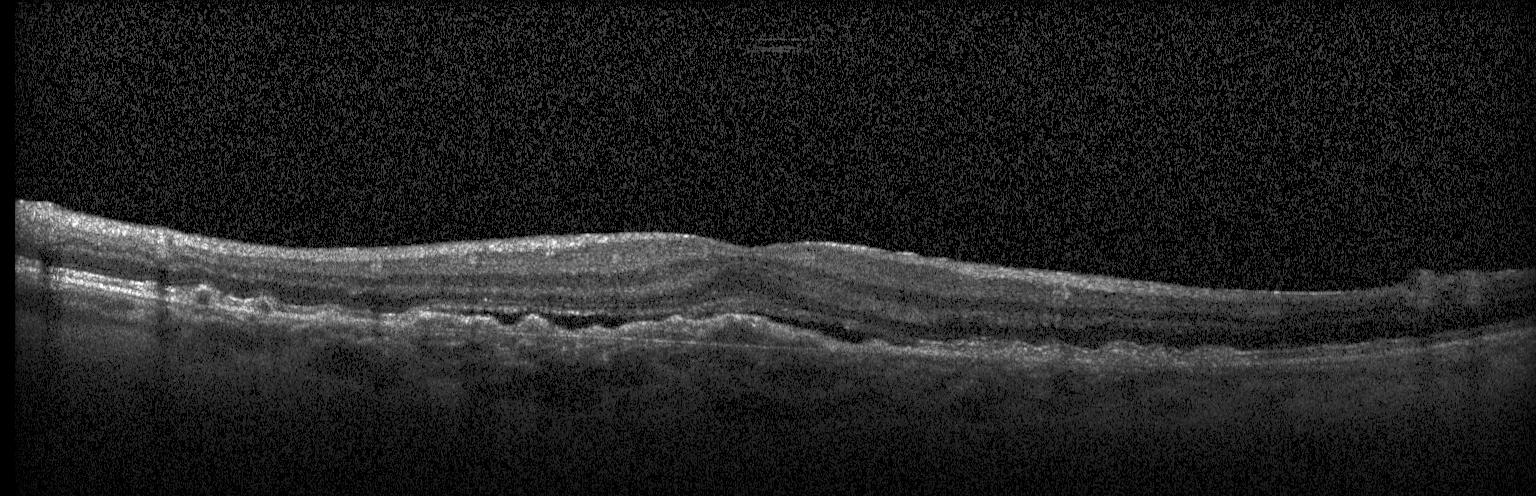
Through the macula; SD-OCT; optical coherence tomography B-scan; Heidelberg Spectralis
Finding: a choroidal neovascular membrane.